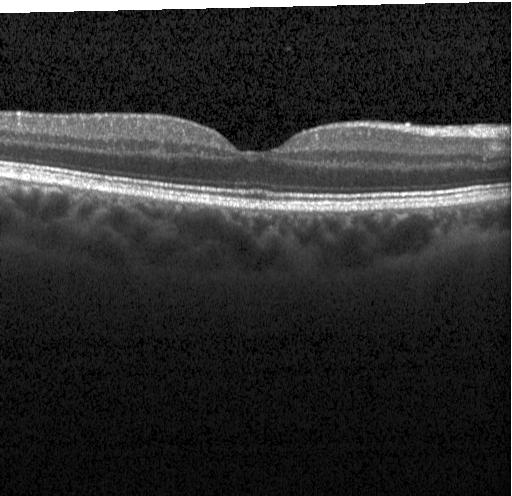

Optical coherence tomography scan.
Impression: neither choroidal neovascularization, diabetic macular edema, nor drusen.